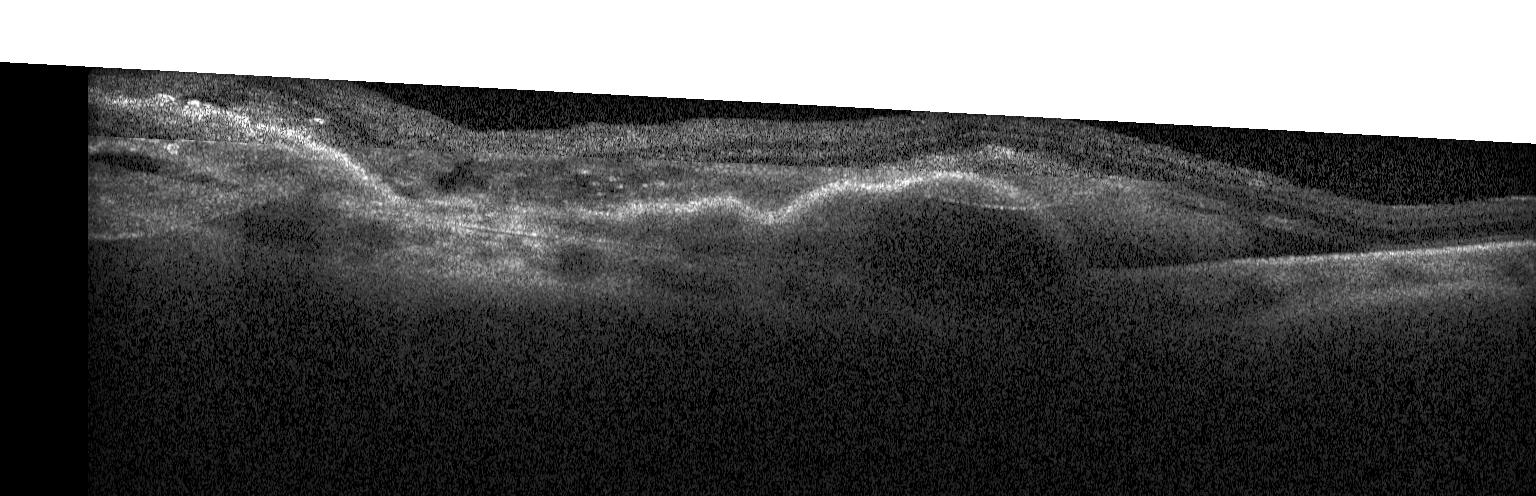

Diagnosis: a choroidal neovascular membrane.